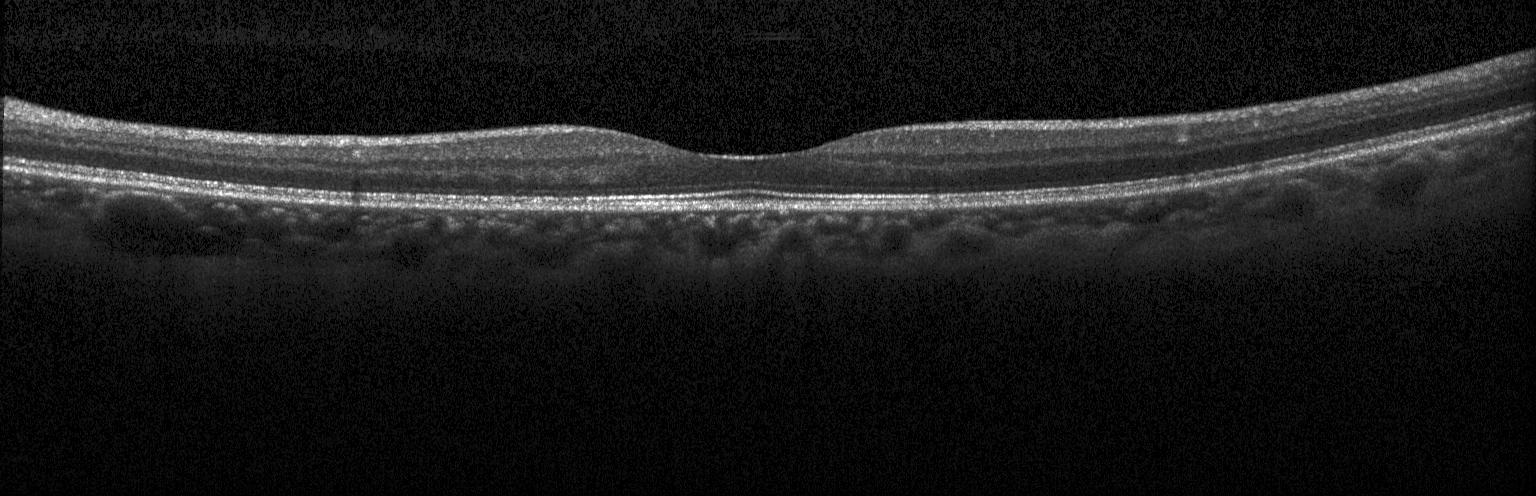

Macular OCT demonstrating no choroidal neovascularization, no diabetic macular edema, and no drusen.